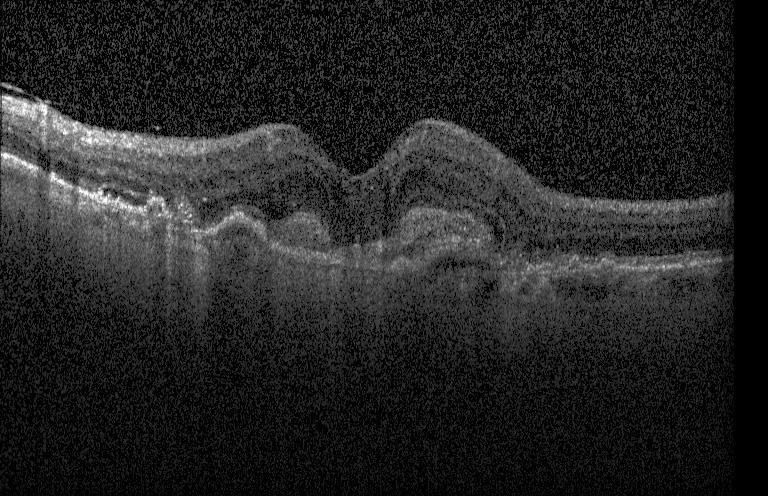 Heidelberg Spectralis. Macular scan. Spectral-domain OCT. Optical coherence tomography scan
The scan shows choroidal neovascularization (CNV).